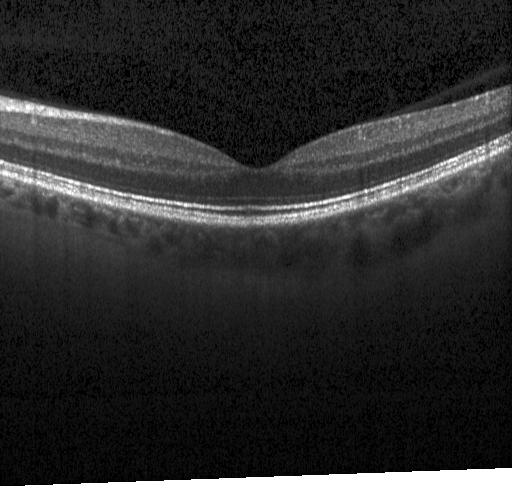

OCT B-scan showing no CNV, no DME, and no drusen.